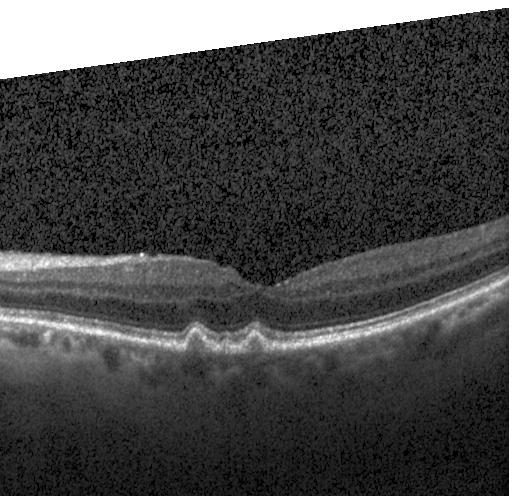
Spectral-domain OCT, optical coherence tomography scan. Finding: sub-RPE drusenoid deposits.